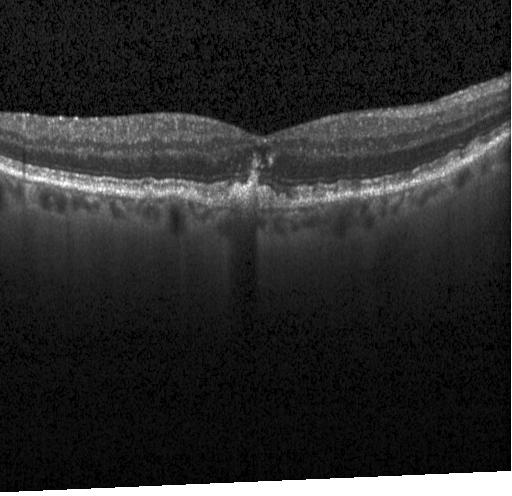

Acquired on a Heidelberg Spectralis · spectral-domain OCT · optical coherence tomography scan · horizontal scan through the fovea.
Diagnosis: drusen.